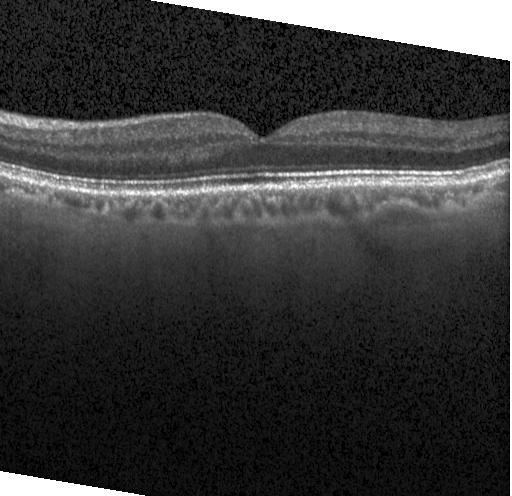 Heidelberg Spectralis OCT system; OCT B-scan; centered on the fovea — Diagnosis: neither choroidal neovascularization, diabetic macular edema, nor drusen.